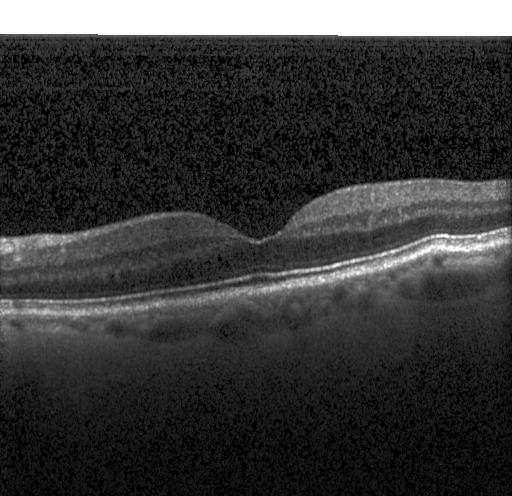
Macular OCT: neither choroidal neovascularization, diabetic macular edema, nor drusen.